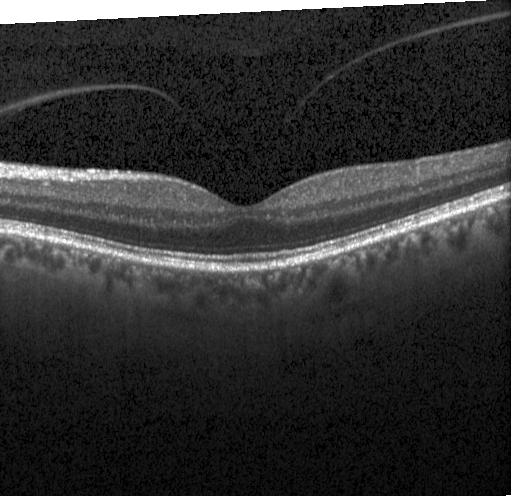 Optical coherence tomography scan · acquired on a Heidelberg Spectralis. Diagnosis: neither CNV, DME, nor drusen.